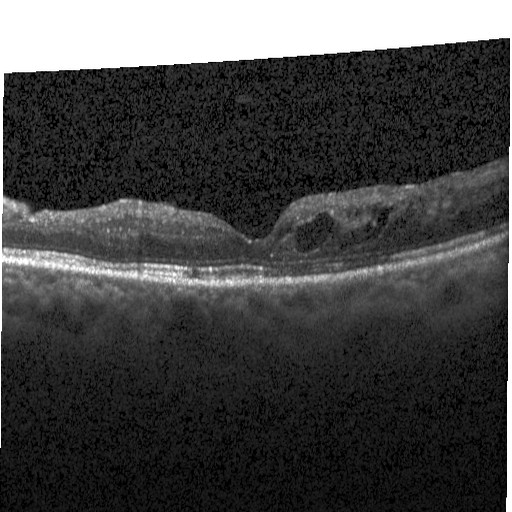 Finding: diabetic macular edema (DME).